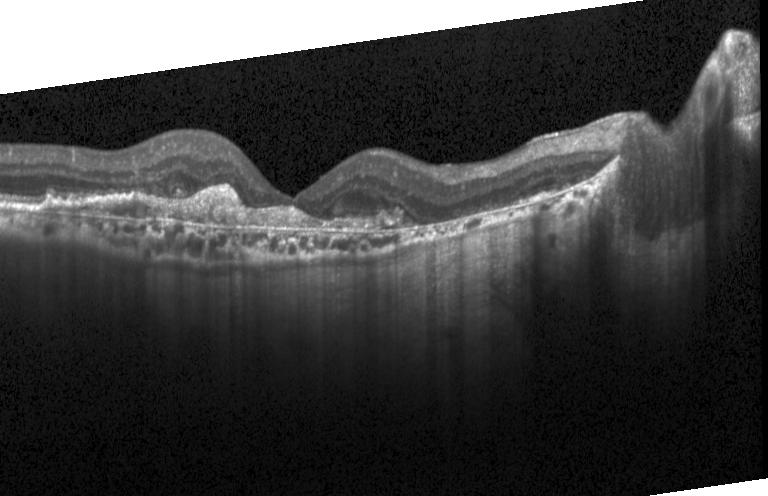

OCT B-scan showing a choroidal neovascular membrane.